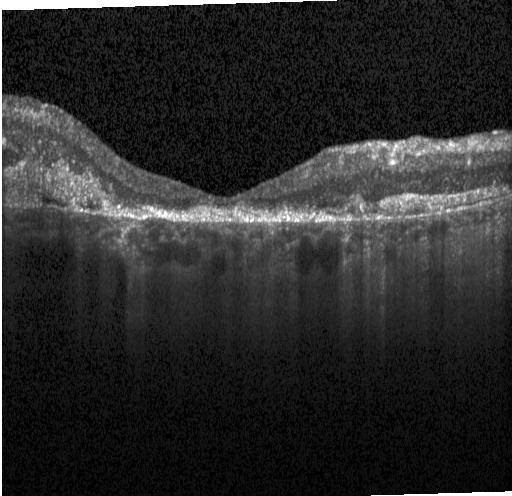 Spectral-domain OCT; Heidelberg Spectralis; macular scan; optical coherence tomography scan
This B-scan demonstrates a choroidal neovascular membrane.